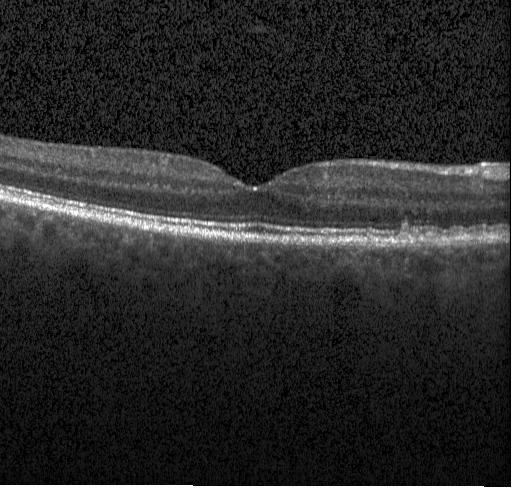 Optical coherence tomography scan.
Impression: drusen.